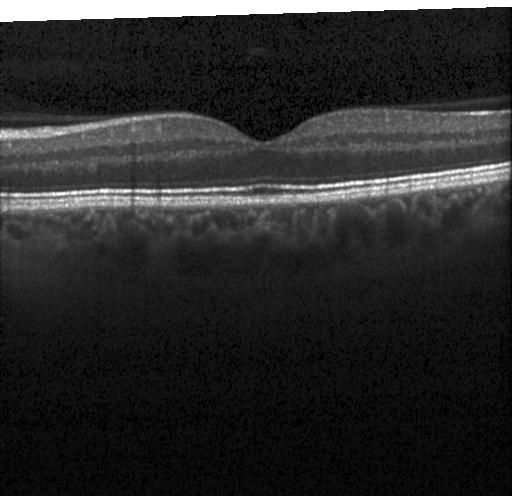

Diagnosis: no choroidal neovascularization, diabetic macular edema, or drusen.